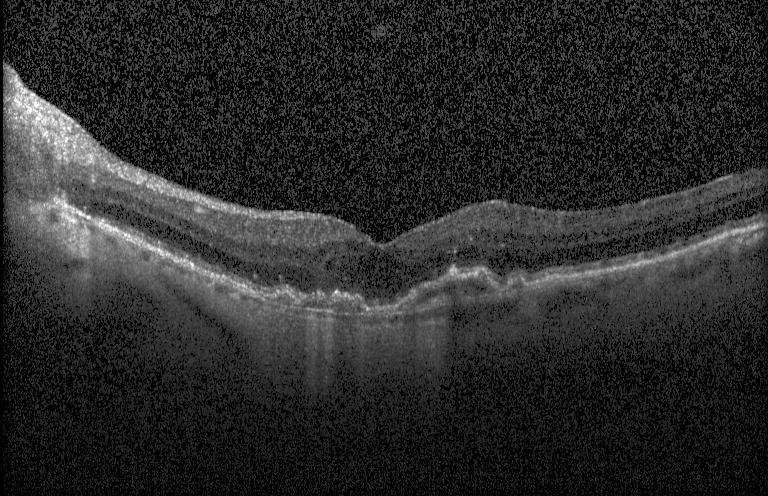 Spectral-domain OCT B-scan: choroidal neovascularization (CNV).